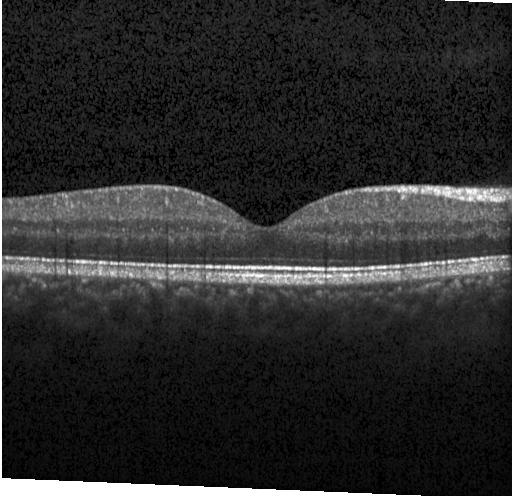

The scan shows neither choroidal neovascularization, diabetic macular edema, nor drusen.